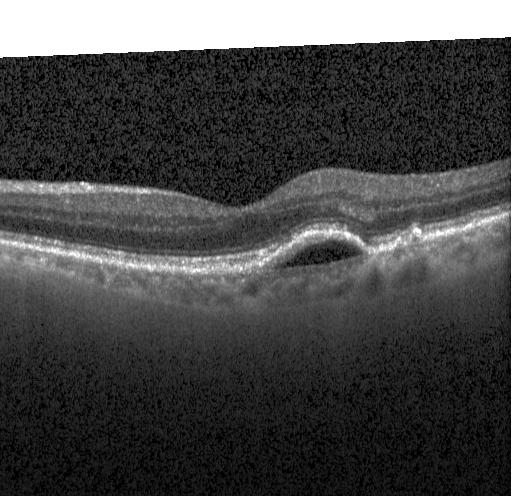

Acquired on a Heidelberg Spectralis, spectral-domain OCT, centered on the fovea, OCT B-scan.
Impression: a choroidal neovascular membrane.